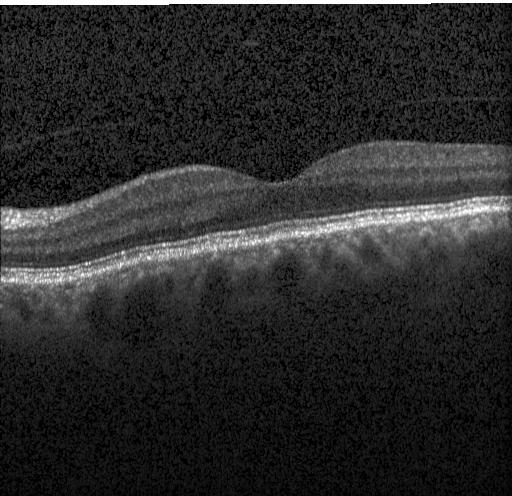
OCT B-scan. Assessment: neither CNV, DME, nor drusen.